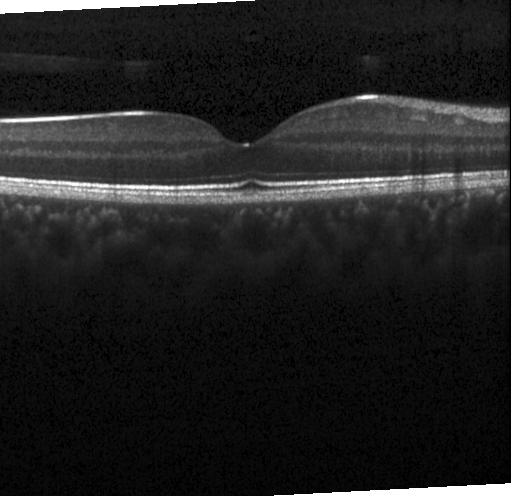

Spectral-domain OCT · OCT line scan — Diagnosis: no evidence of choroidal neovascularization, diabetic macular edema, or drusen.